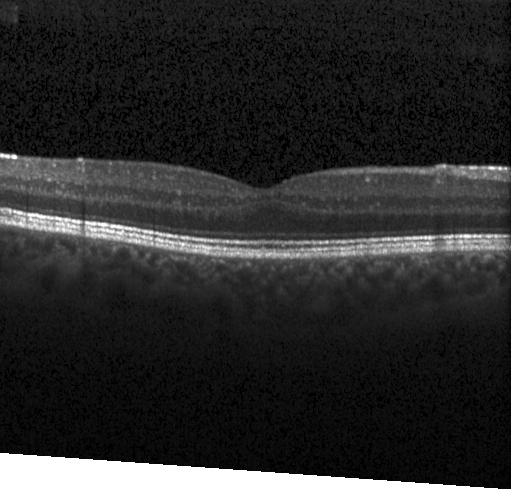
Spectral-domain optical coherence tomography, OCT line scan. Impression: no choroidal neovascularization, diabetic macular edema, or drusen.